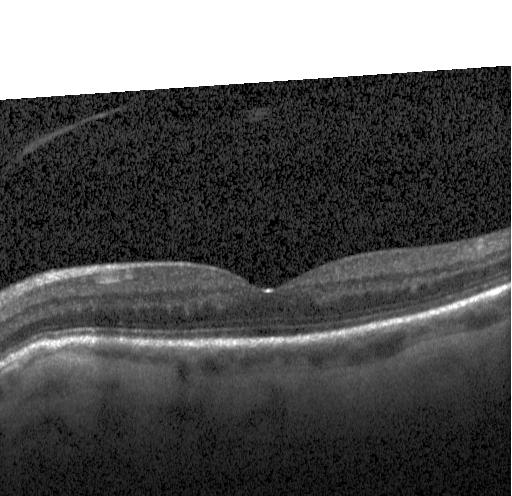 Spectral-domain optical coherence tomography; retinal OCT B-scan.
Finding: neither CNV, DME, nor drusen.